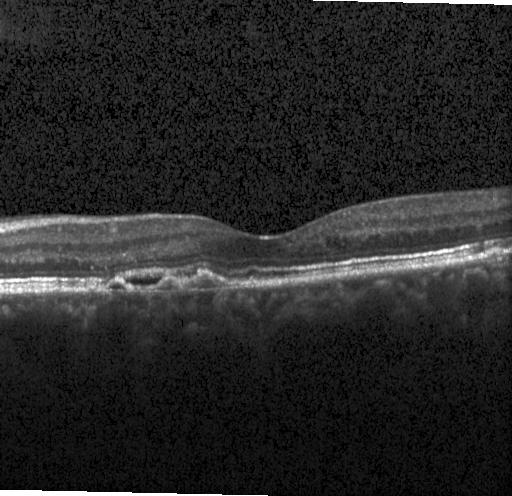
This B-scan demonstrates CNV.